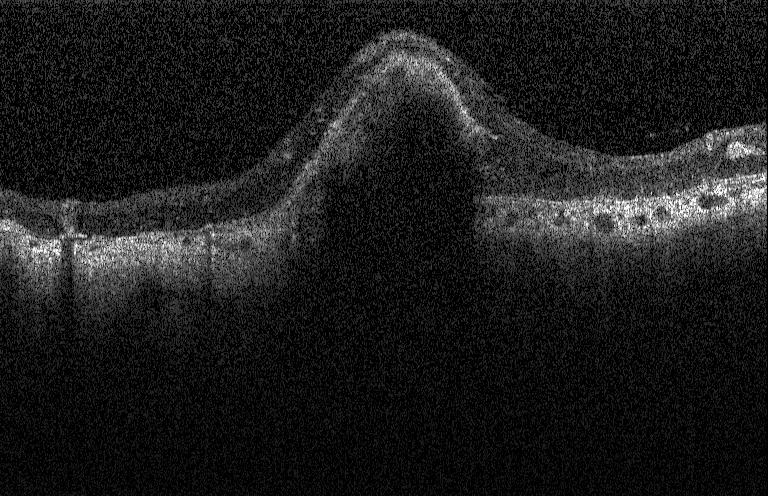 Diagnosis: a choroidal neovascular membrane.